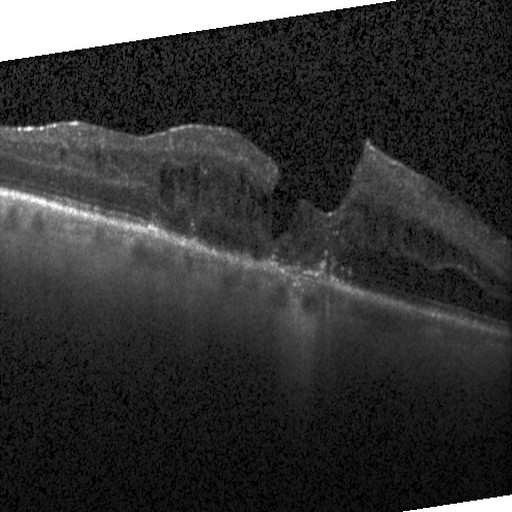

Spectral-domain OCT B-scan: diabetic macular edema.